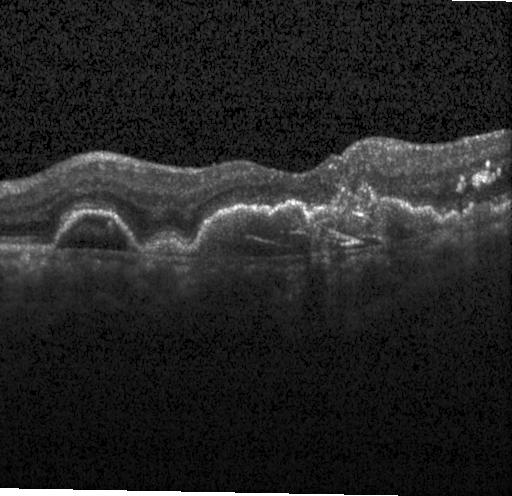

Optical coherence tomography scan — Macular OCT: choroidal neovascularization (CNV).